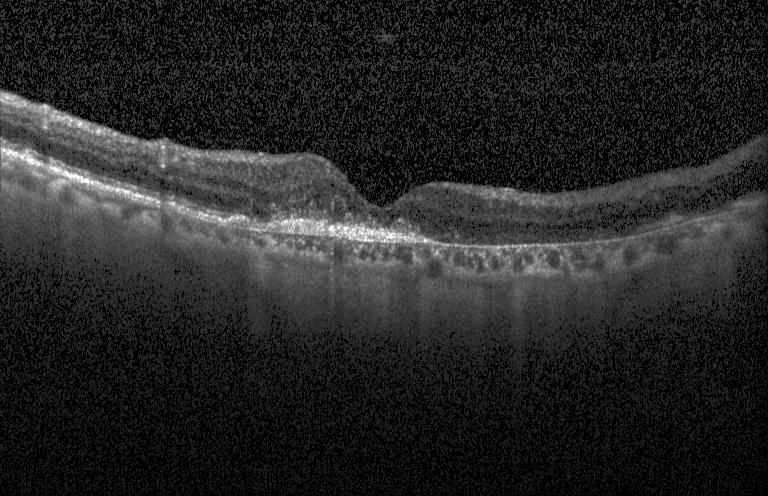
OCT B-scan. Finding: CNV.